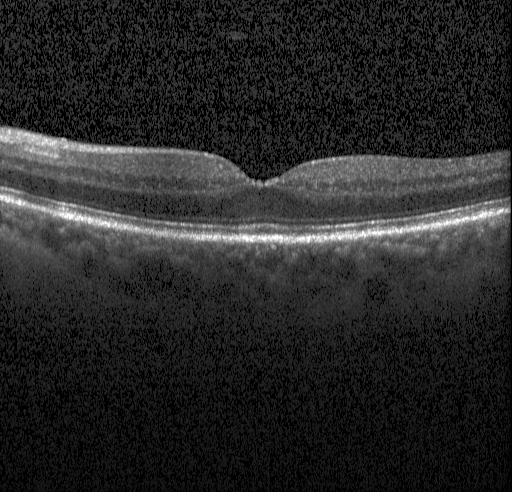

Acquired on a Heidelberg Spectralis; spectral-domain OCT; optical coherence tomography B-scan. Dx: neither choroidal neovascularization, diabetic macular edema, nor drusen.